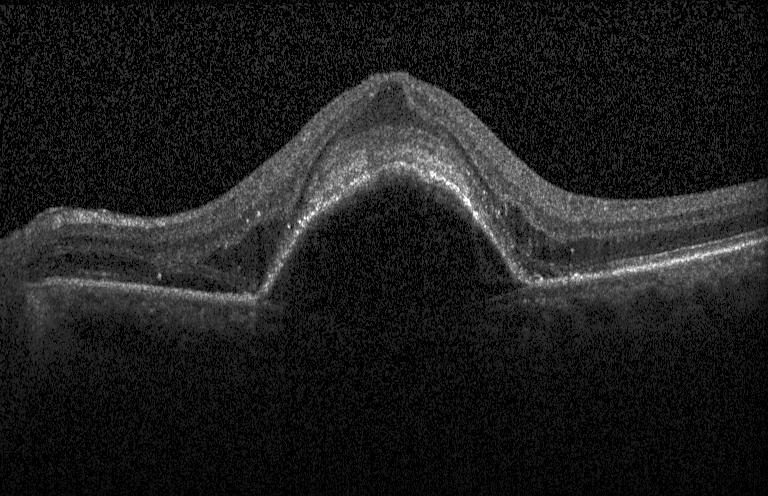

The scan shows a choroidal neovascular membrane.